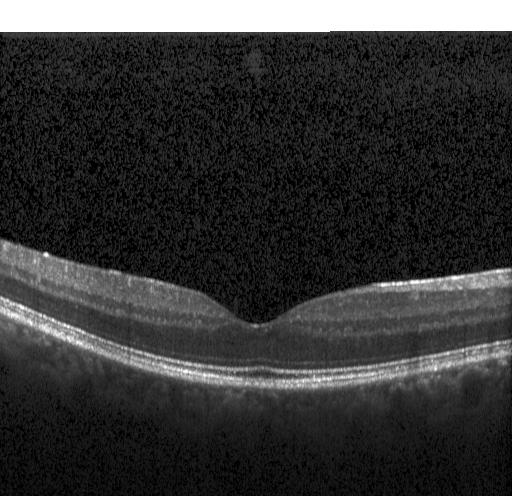 Spectral-domain optical coherence tomography; retinal OCT cross-section. Neither choroidal neovascularization, diabetic macular edema, nor drusen.